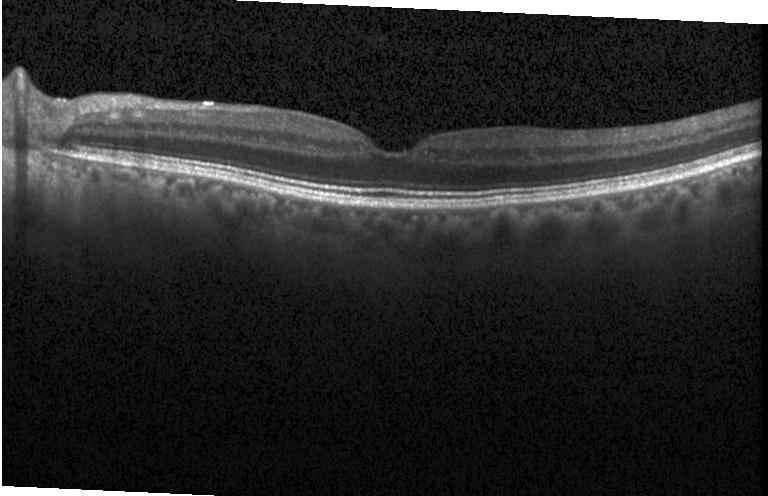 SD-OCT · retinal OCT B-scan · instrument: Heidelberg Spectralis · macular scan
This B-scan demonstrates no choroidal neovascularization, no diabetic macular edema, and no drusen.